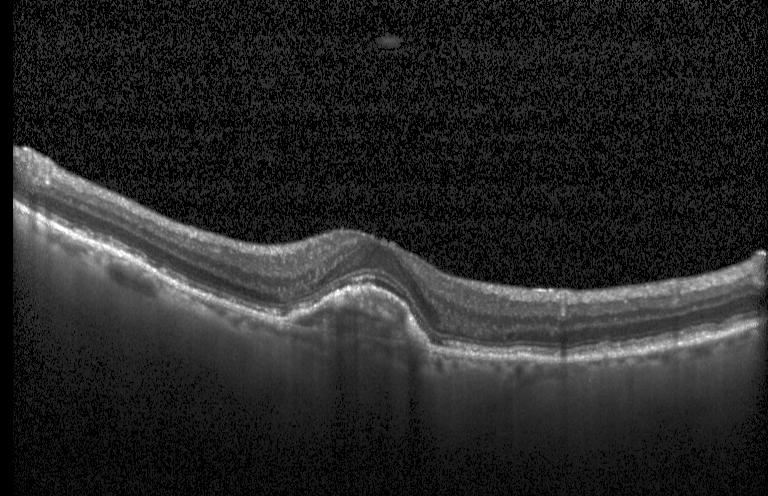
Dx: a choroidal neovascular membrane.